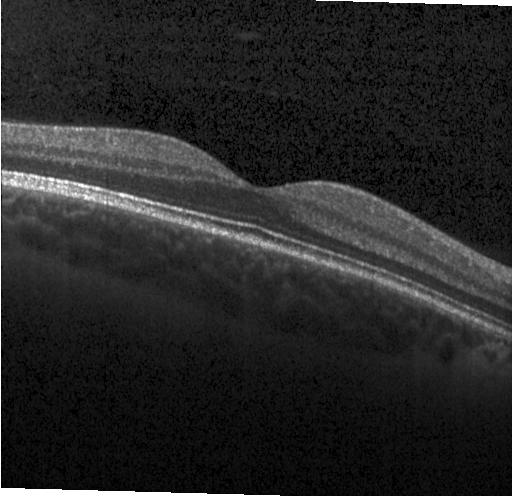
Optical coherence tomography B-scan. No CNV, DME, or drusen.